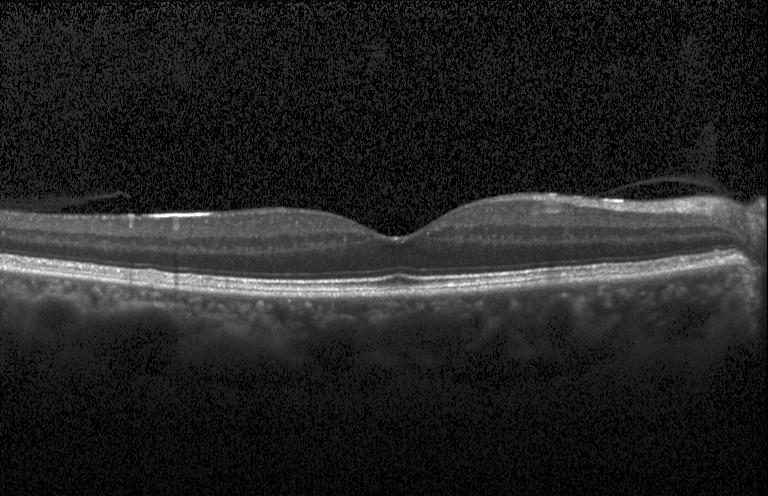

OCT finding: no evidence of CNV, DME, or drusen.